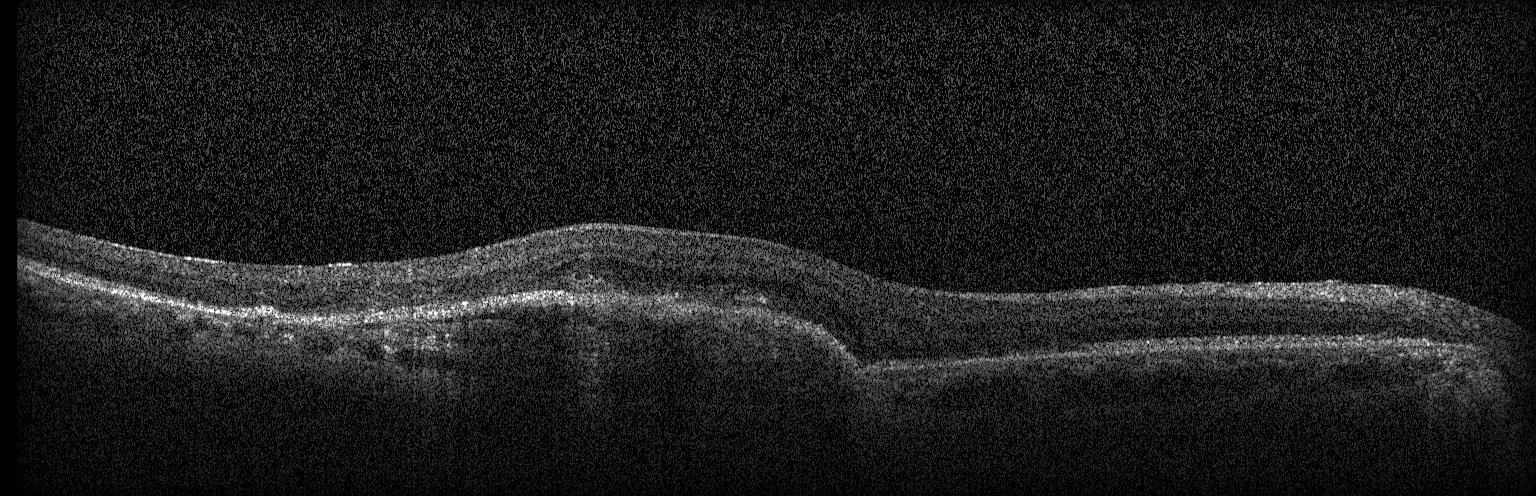 The scan shows a choroidal neovascular membrane.